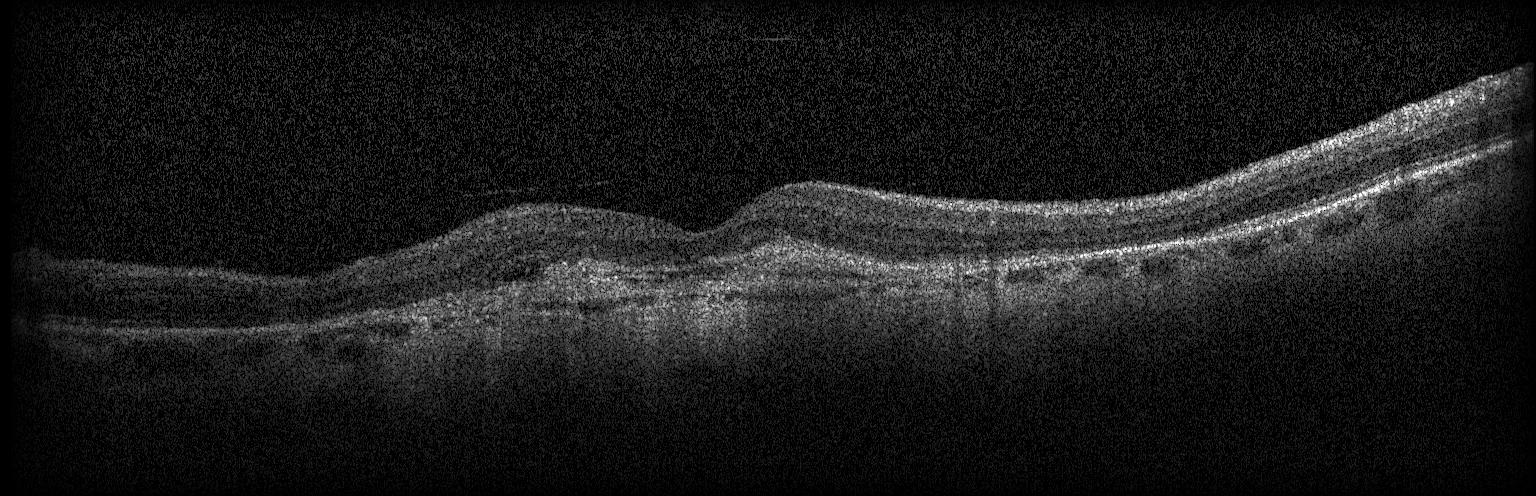

Retinal OCT B-scan. Acquired on a Heidelberg Spectralis.
The scan shows choroidal neovascularization (CNV).